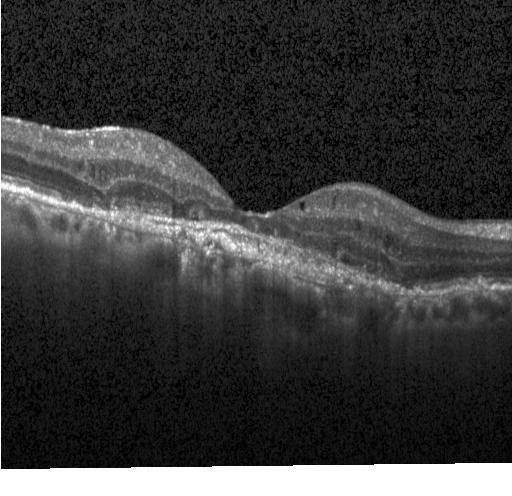 Macular scan, OCT line scan, spectral-domain optical coherence tomography
A choroidal neovascular membrane.